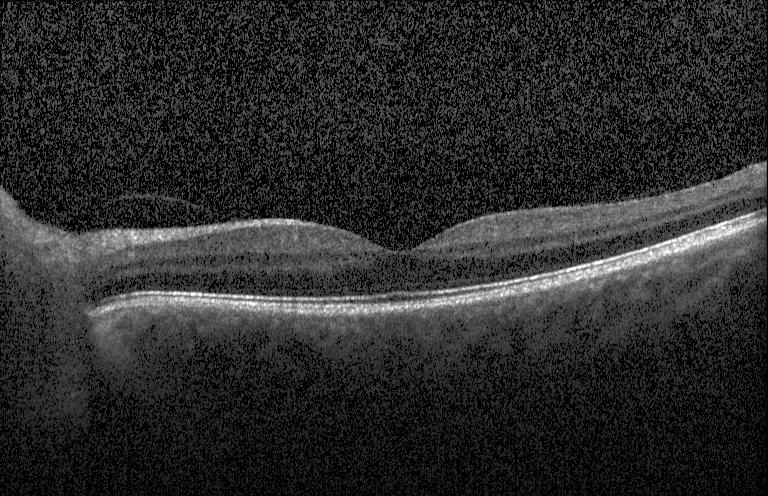
Heidelberg Spectralis; through the macula; OCT B-scan.
No choroidal neovascularization, no diabetic macular edema, and no drusen.